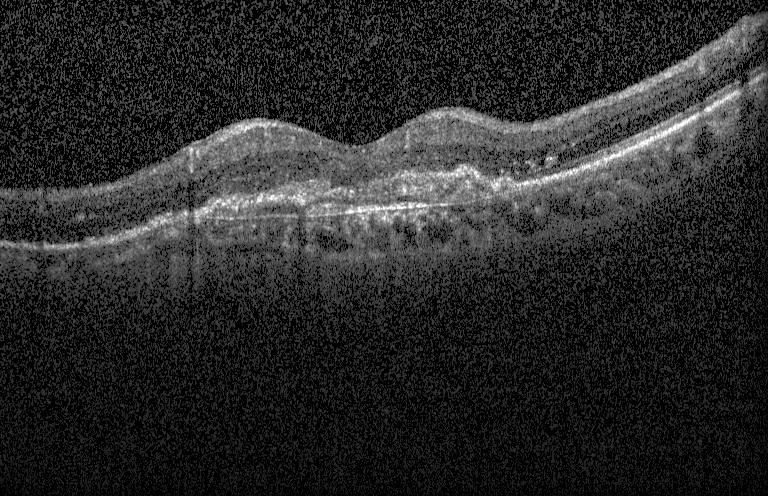
Assessment: a choroidal neovascular membrane.